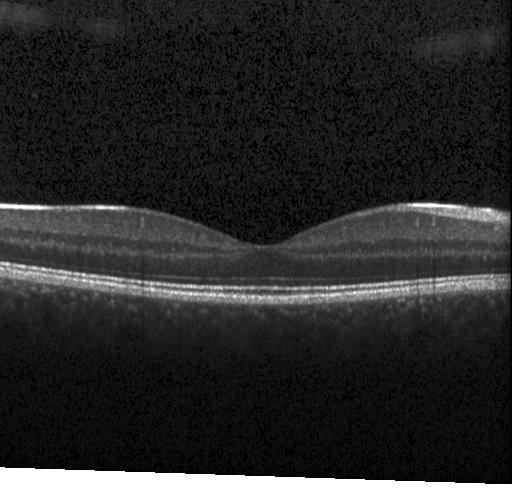
Macular OCT demonstrating neither choroidal neovascularization, diabetic macular edema, nor drusen.